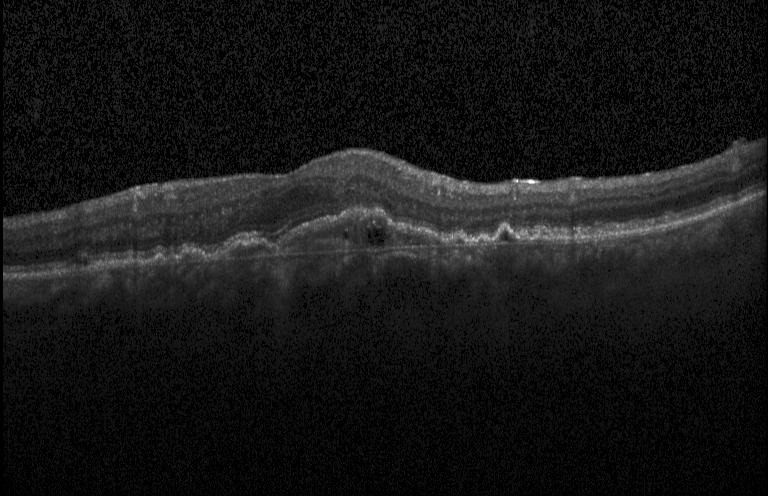
Impression: a choroidal neovascular membrane.